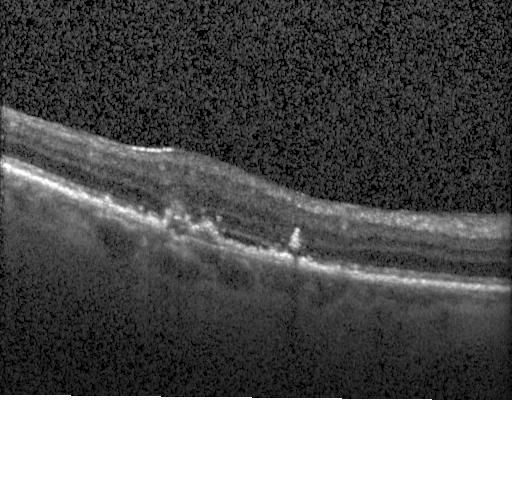
Finding: choroidal neovascularization.